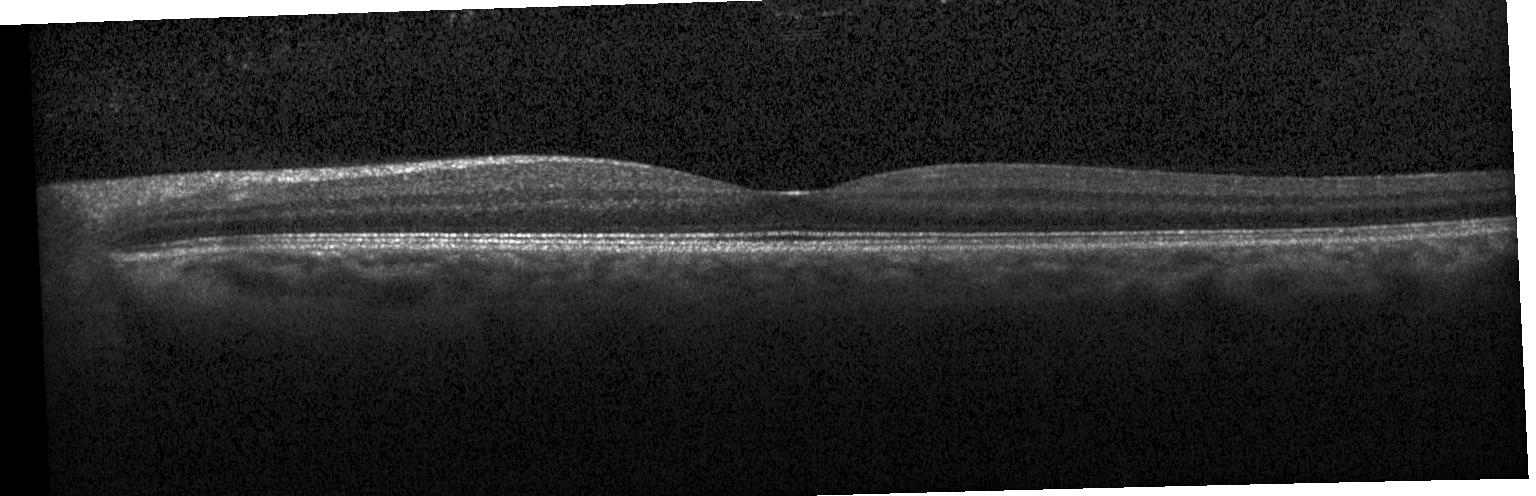
Macular OCT demonstrating neither choroidal neovascularization, diabetic macular edema, nor drusen.